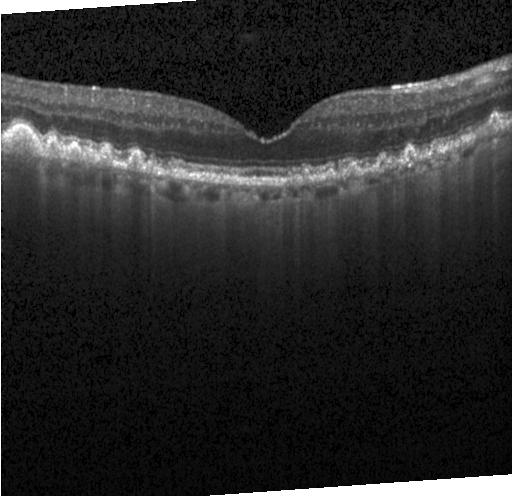

Optical coherence tomography scan. Instrument: Heidelberg Spectralis. Horizontal scan through the fovea
Assessment: multiple drusen.